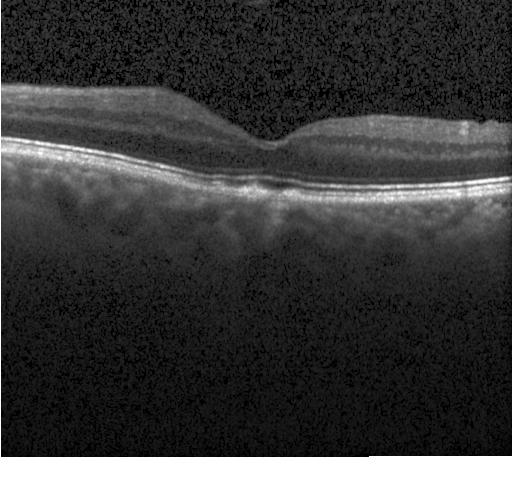 Impression: sub-RPE drusenoid deposits.